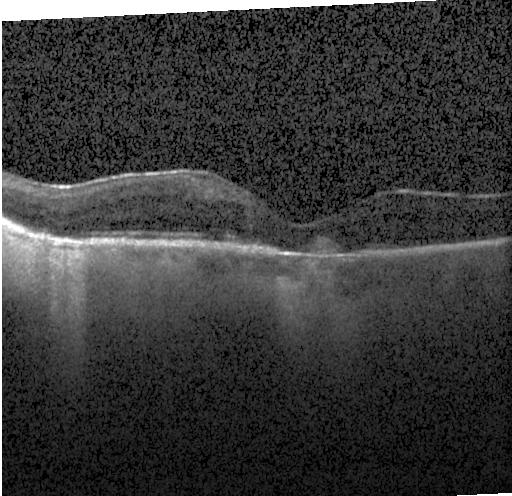
Finding: a choroidal neovascular membrane.